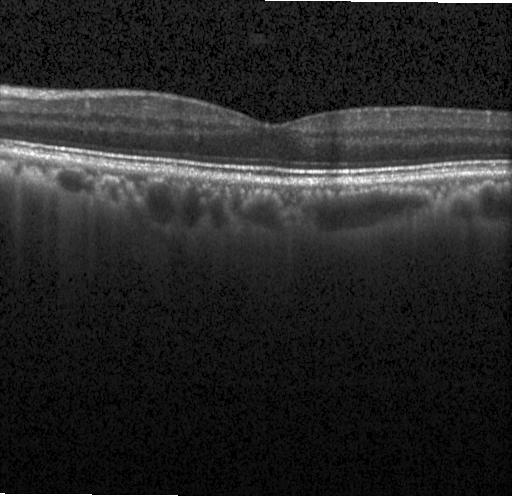

Dx: no choroidal neovascularization, diabetic macular edema, or drusen.